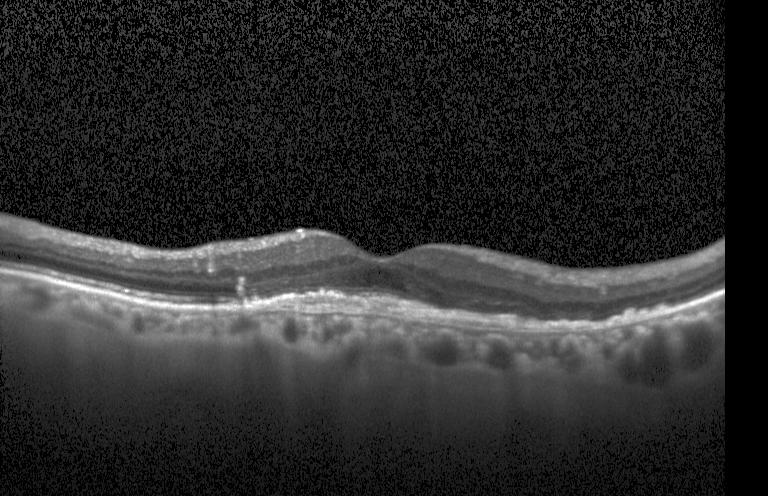

OCT B-scan. Impression: a choroidal neovascular membrane.